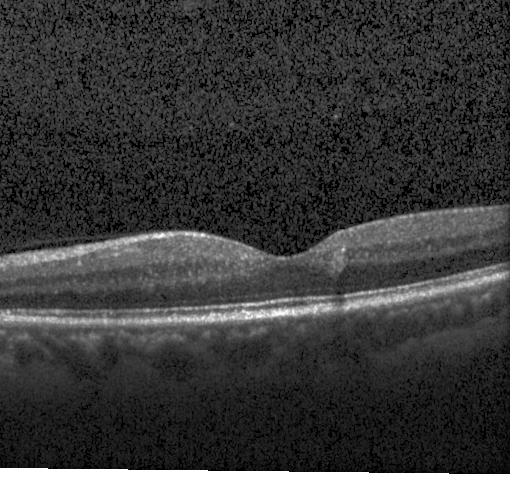
Macular scan · retinal OCT B-scan · instrument: Heidelberg Spectralis — Diagnosis: no evidence of choroidal neovascularization, diabetic macular edema, or drusen.